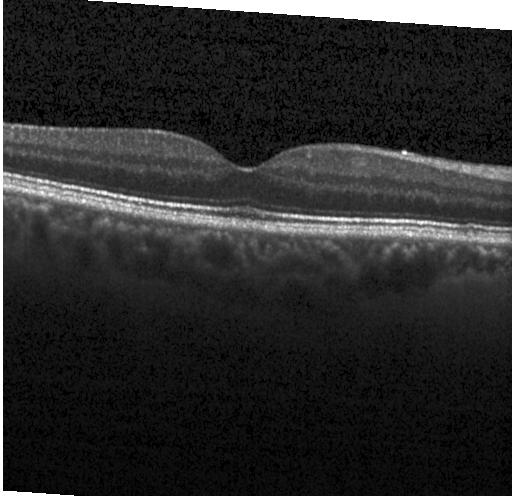
OCT finding: no CNV, no DME, and no drusen.